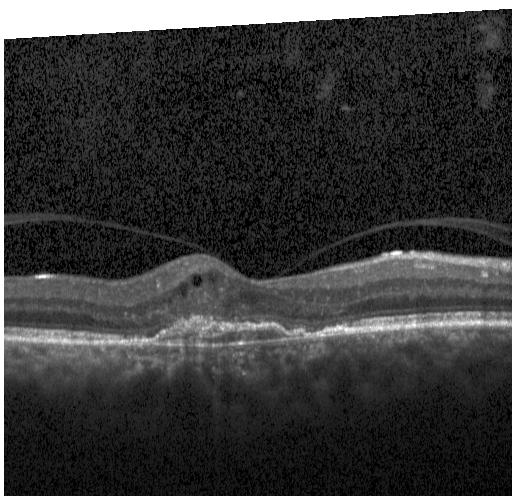 Spectral-domain optical coherence tomography, optical coherence tomography B-scan — Impression: choroidal neovascularization (CNV).